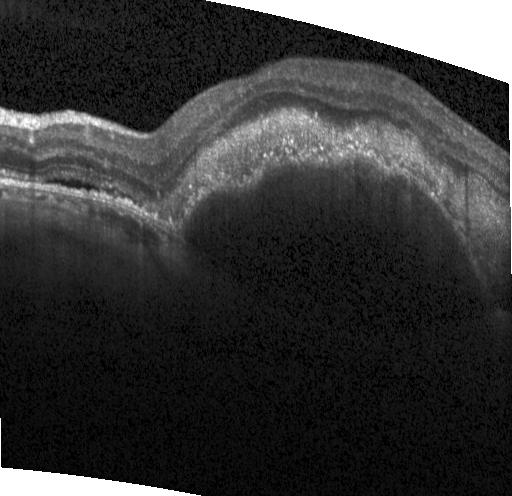
This B-scan demonstrates CNV.